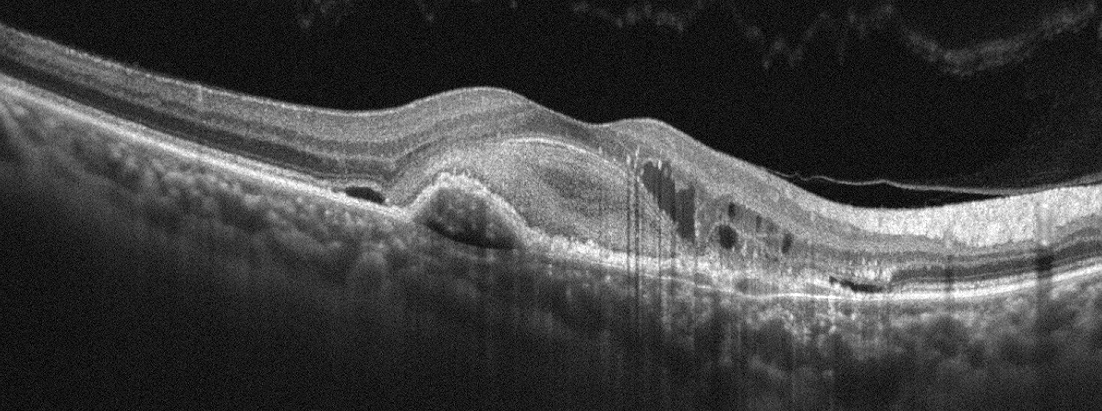 Macular OCT demonstrating age-related macular degeneration.